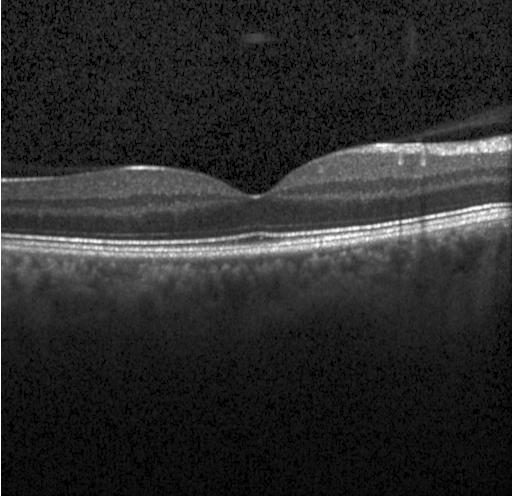 Spectral-domain OCT; retinal OCT B-scan.
Assessment: neither choroidal neovascularization, diabetic macular edema, nor drusen.